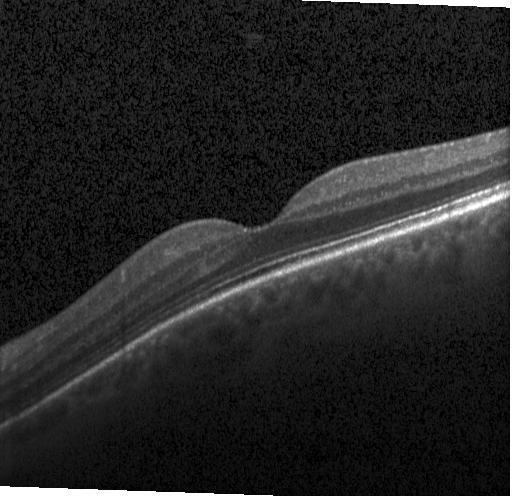
Optical coherence tomography scan
OCT finding: no evidence of CNV, DME, or drusen.